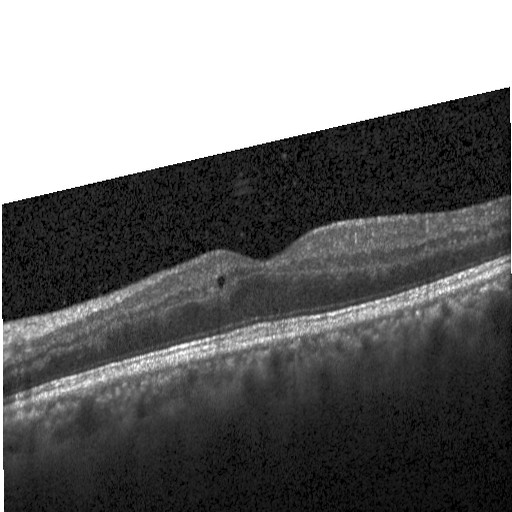
OCT finding: diabetic macular edema (DME).